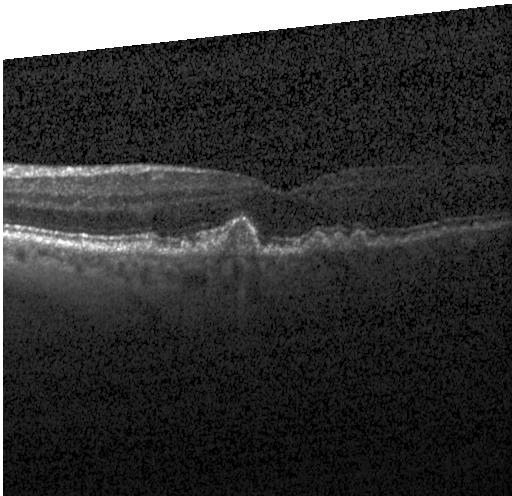
Centered on the fovea. Optical coherence tomography B-scan. Heidelberg Spectralis OCT system. Finding: multiple drusen.